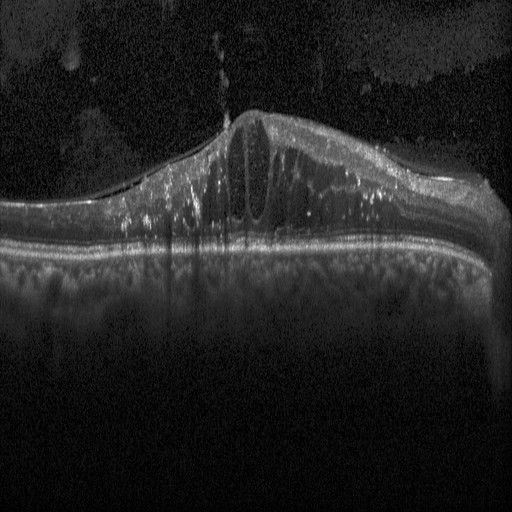
OCT line scan, macular scan
Diagnosis: DME.